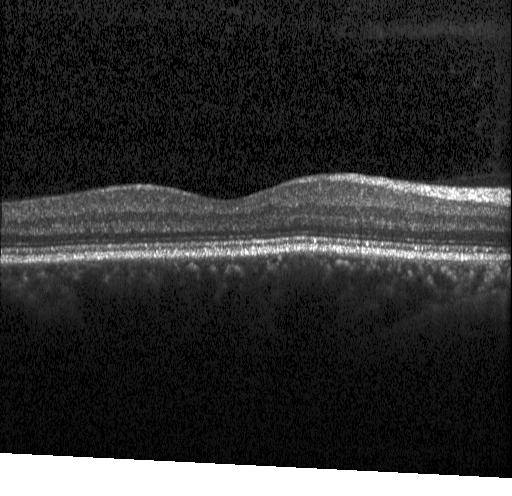
Retinal OCT cross-section, spectral-domain optical coherence tomography, centered on the fovea, instrument: Heidelberg Spectralis.
Impression: no choroidal neovascularization, diabetic macular edema, or drusen.